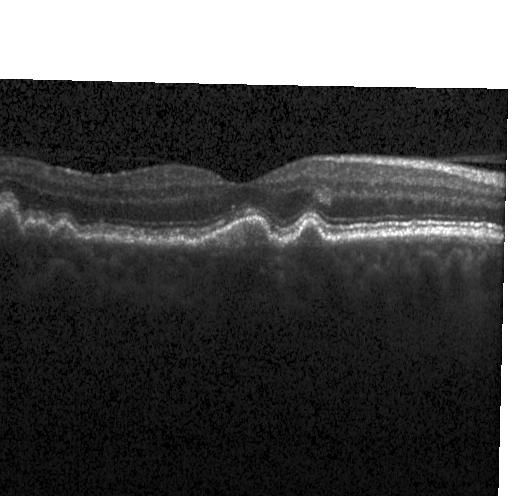 The scan shows multiple drusen.